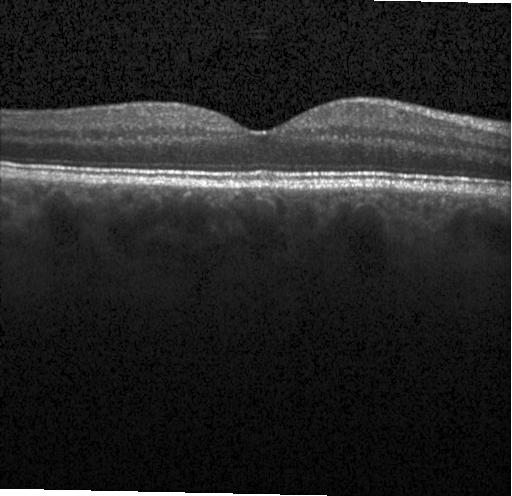 Retinal OCT cross-section; Heidelberg Spectralis OCT system; macular scan
The scan shows no choroidal neovascularization, no diabetic macular edema, and no drusen.